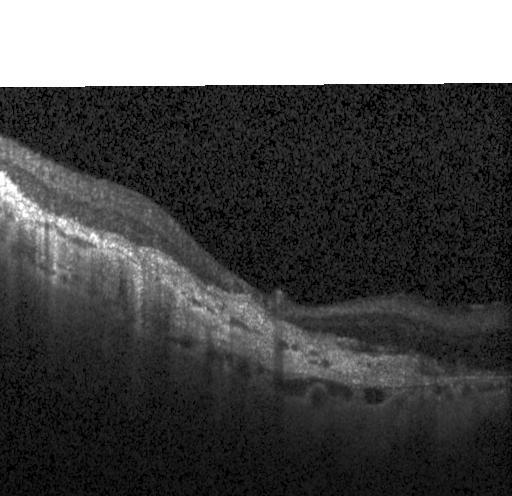 Diagnosis: a choroidal neovascular membrane.